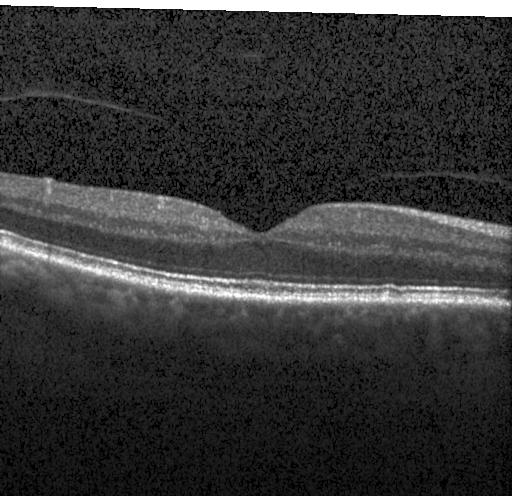 Heidelberg Spectralis · fovea-centered · spectral-domain OCT · OCT line scan. Finding: neither CNV, DME, nor drusen.